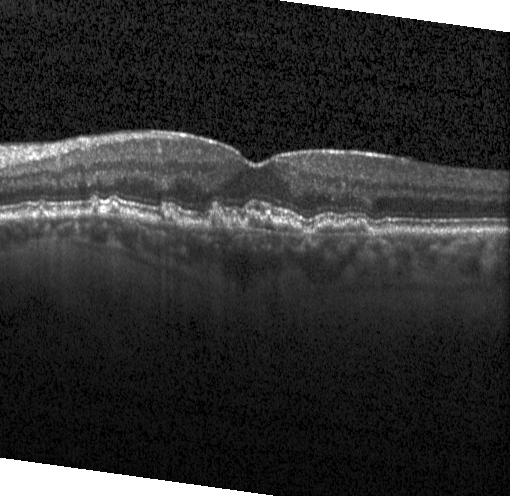
Macular OCT: drusen.